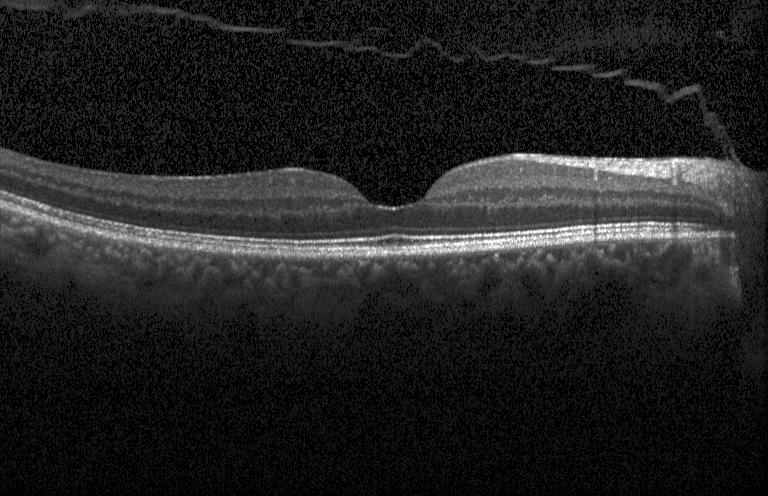 Retinal OCT cross-section.
The scan shows neither CNV, DME, nor drusen.